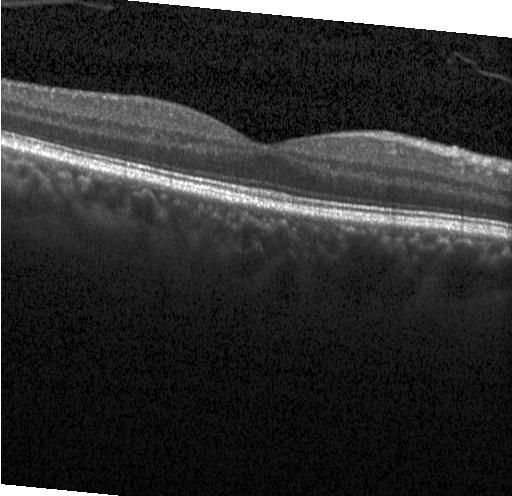 Acquired on a Heidelberg Spectralis. Horizontal scan through the fovea. OCT B-scan — OCT finding: no evidence of choroidal neovascularization, diabetic macular edema, or drusen.